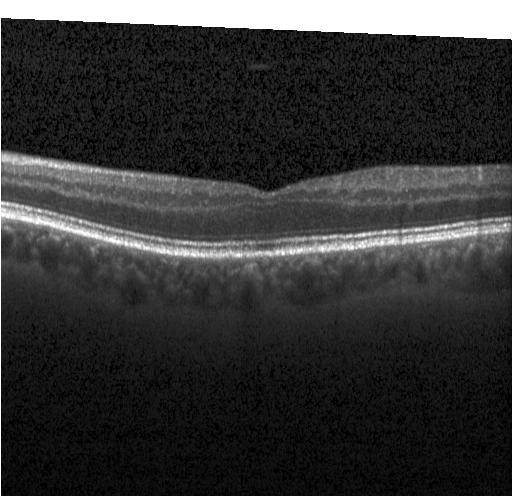
SD-OCT, acquired on a Heidelberg Spectralis, fovea-centered, optical coherence tomography scan.
Diagnosis: no evidence of CNV, DME, or drusen.